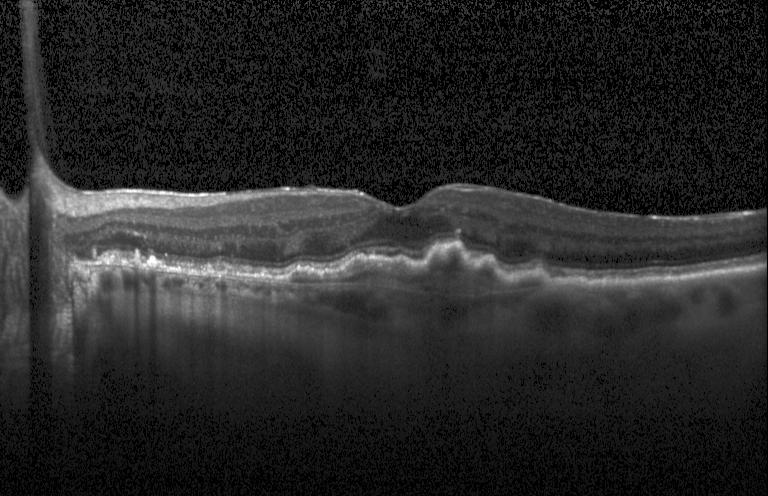
Retinal OCT B-scan.
Dx: choroidal neovascularization.